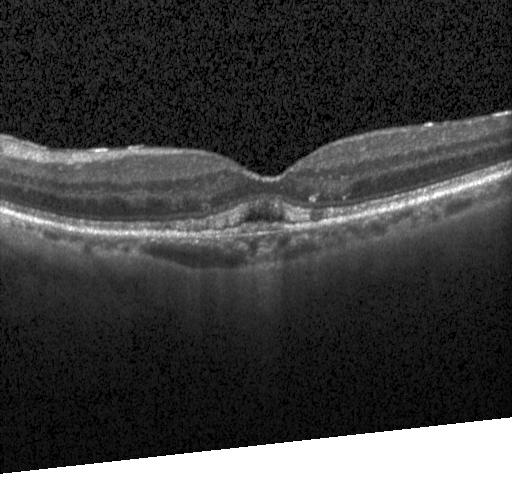

Instrument: Heidelberg Spectralis · fovea-centered · spectral-domain OCT · retinal OCT B-scan. Impression: choroidal neovascularization.